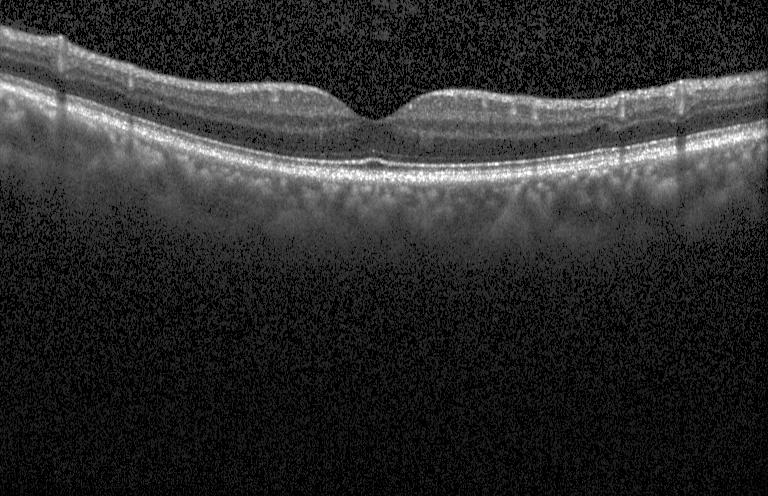 OCT B-scan. SD-OCT. Macular scan. Impression: neither CNV, DME, nor drusen.